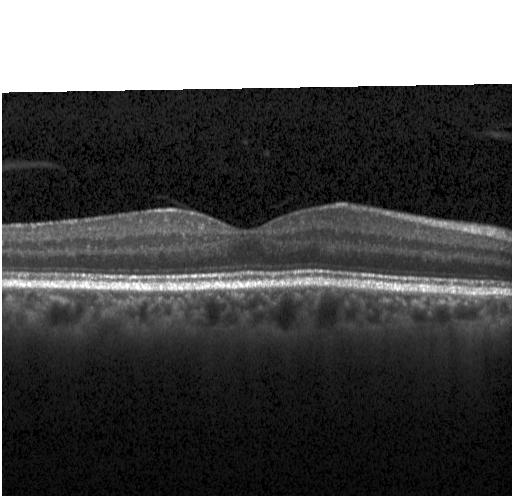 Fovea-centered. OCT B-scan. Heidelberg Spectralis. SD-OCT — OCT finding: no choroidal neovascularization, no diabetic macular edema, and no drusen.